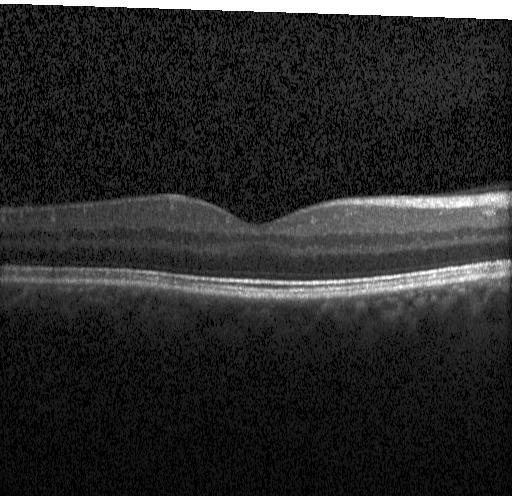
Optical coherence tomography B-scan · spectral-domain OCT · horizontal scan through the fovea — Diagnosis: no choroidal neovascularization, diabetic macular edema, or drusen.